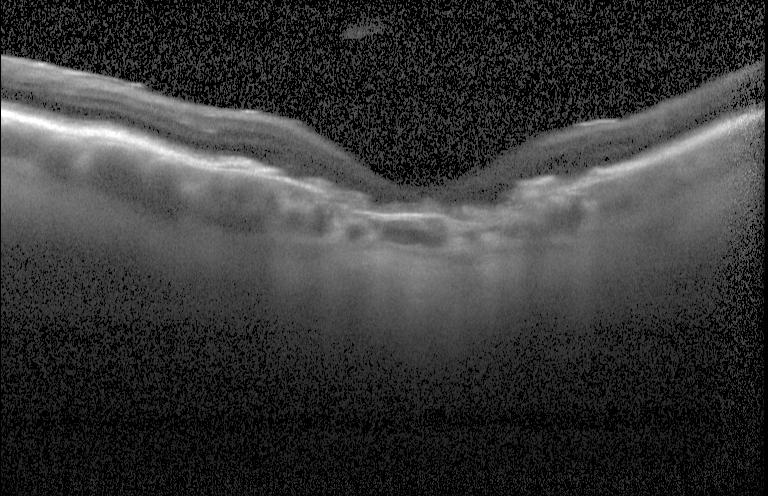
Spectral-domain OCT. Retinal OCT cross-section. Heidelberg Spectralis OCT system. Diagnosis: a choroidal neovascular membrane.